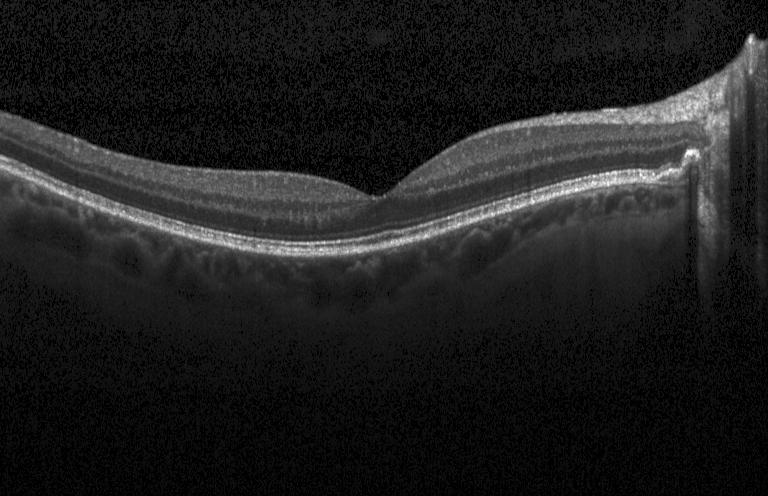
Finding: no choroidal neovascularization, no diabetic macular edema, and no drusen.